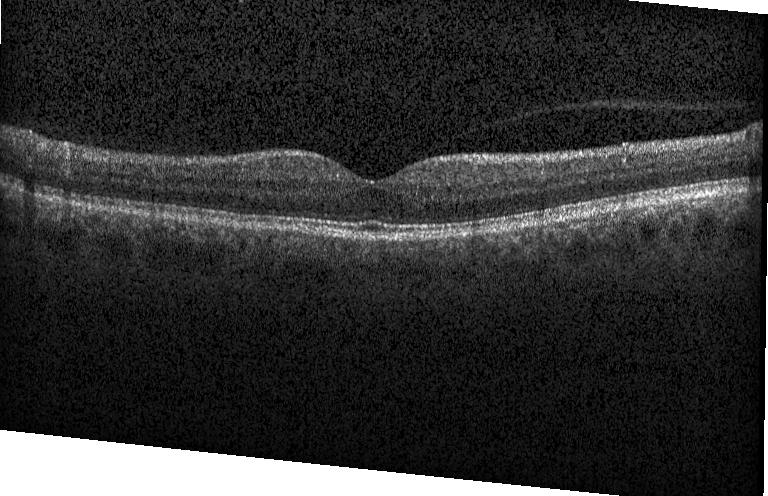 SD-OCT; OCT line scan; Heidelberg Spectralis OCT system; macular scan — Diagnosis: no evidence of choroidal neovascularization, diabetic macular edema, or drusen.